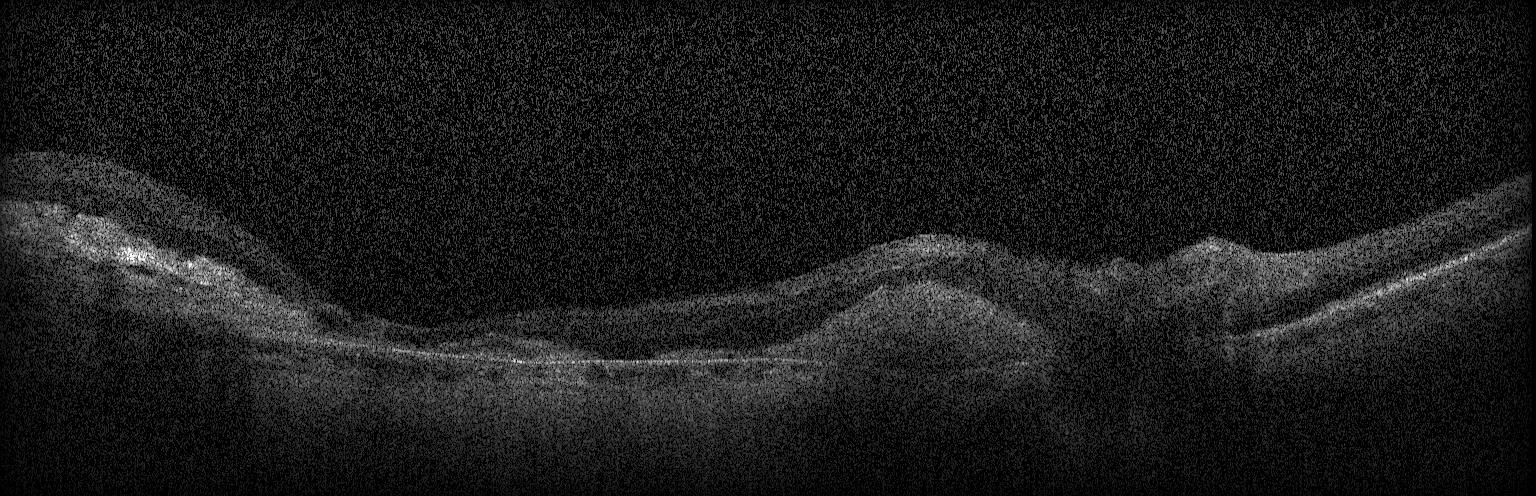
SD-OCT · optical coherence tomography scan — The scan shows choroidal neovascularization (CNV).